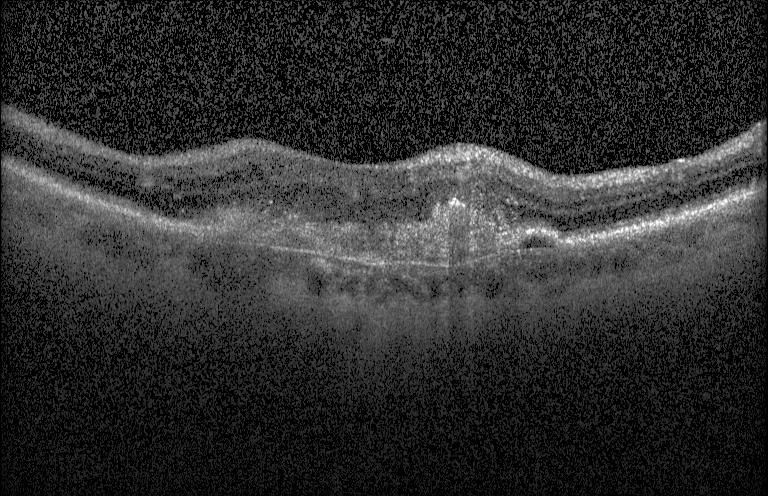 OCT B-scan · acquired on a Heidelberg Spectralis · spectral-domain OCT · through the macula
Impression: a choroidal neovascular membrane.